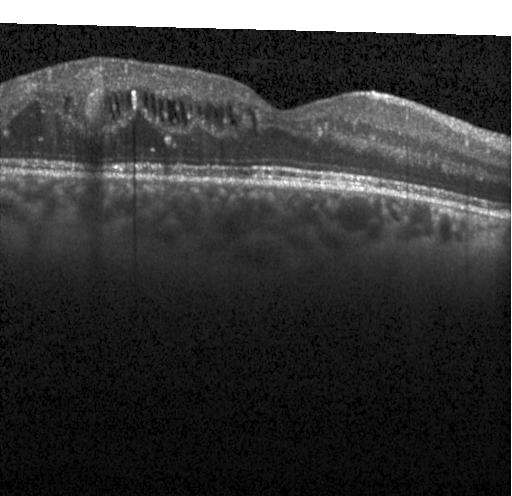 Optical coherence tomography scan. Impression: diabetic macular edema (DME).